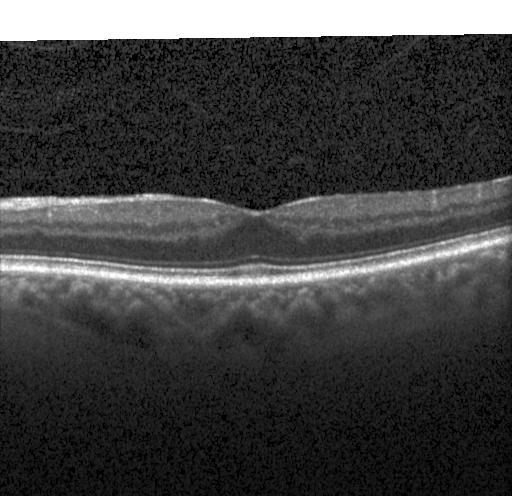 Macular scan. Instrument: Heidelberg Spectralis. Retinal OCT B-scan. This B-scan demonstrates no evidence of choroidal neovascularization, diabetic macular edema, or drusen.